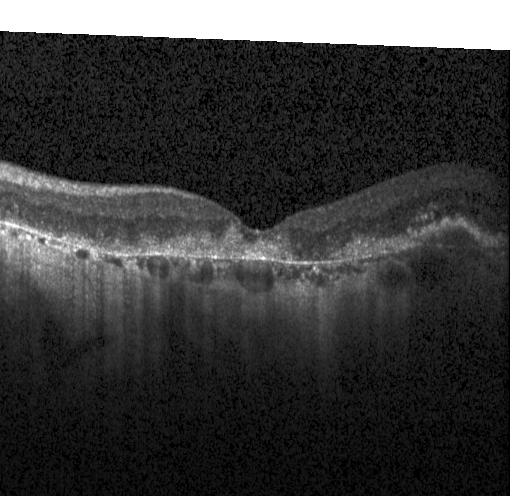

Macular OCT demonstrating a choroidal neovascular membrane.